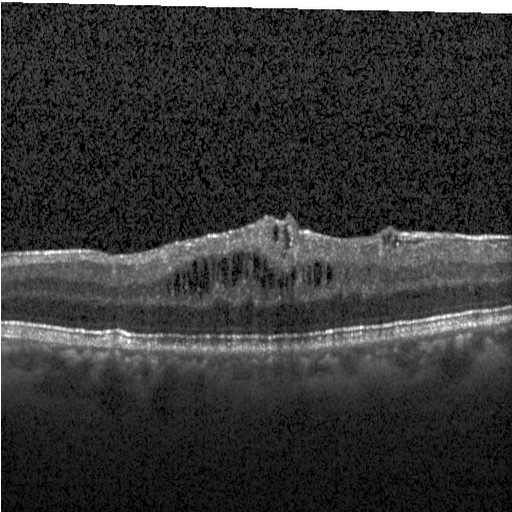

Spectral-domain OCT; horizontal scan through the fovea; OCT line scan — Diabetic macular edema (DME).